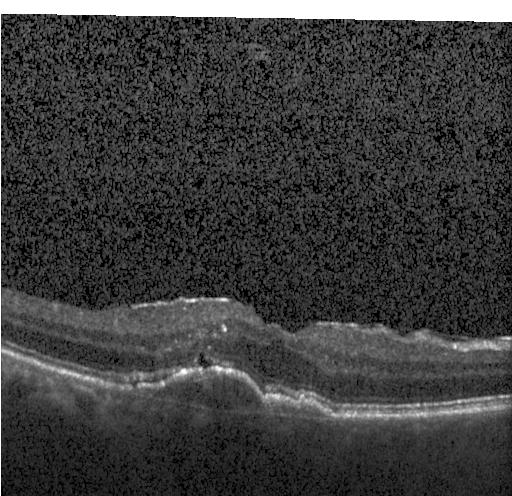

Finding: a choroidal neovascular membrane.